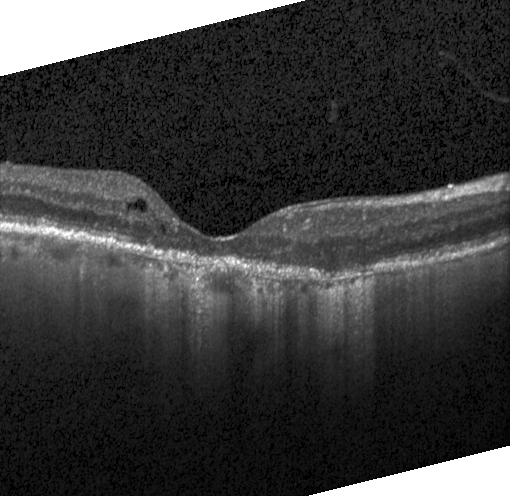 Retinal OCT B-scan. The scan shows a choroidal neovascular membrane.